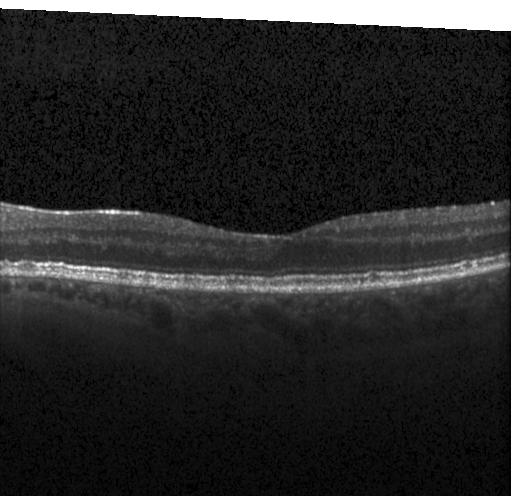

Heidelberg Spectralis OCT system, SD-OCT, optical coherence tomography B-scan.
Diagnosis: neither choroidal neovascularization, diabetic macular edema, nor drusen.